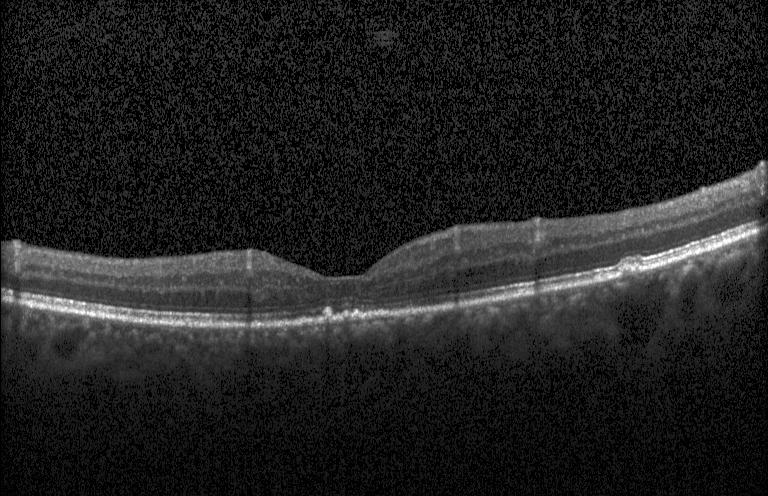
Impression: multiple drusen.